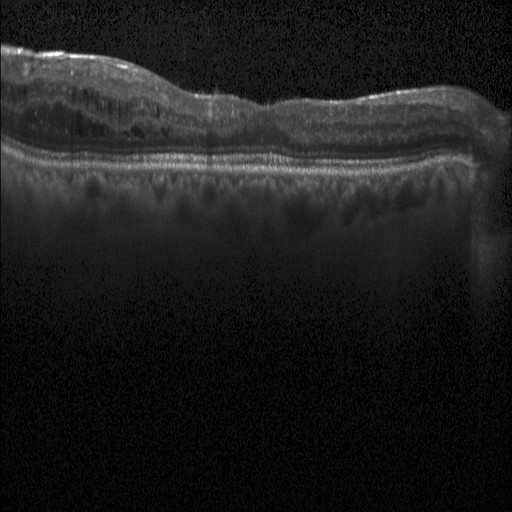

Optical coherence tomography B-scan
Diagnosis: DME.